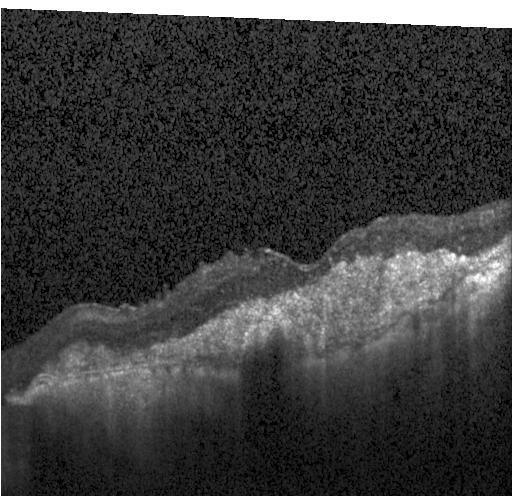 Macular OCT demonstrating CNV.